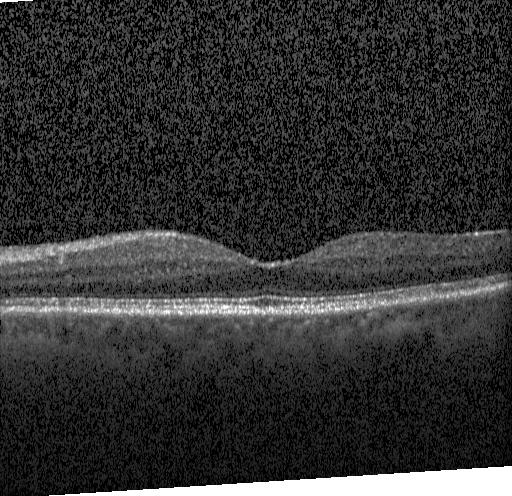

SD-OCT; optical coherence tomography scan; macular scan.
Finding: no CNV, DME, or drusen.